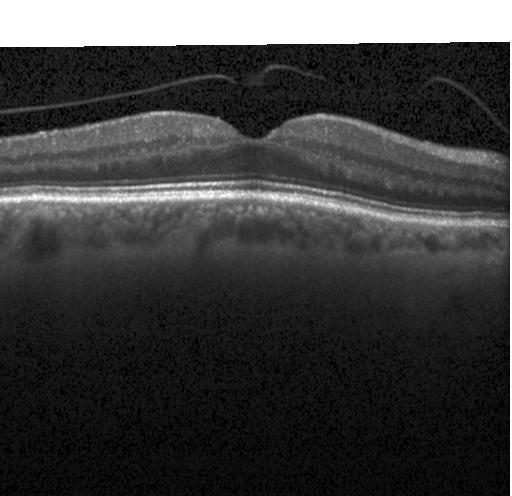

OCT B-scan; spectral-domain OCT
No choroidal neovascularization, diabetic macular edema, or drusen.